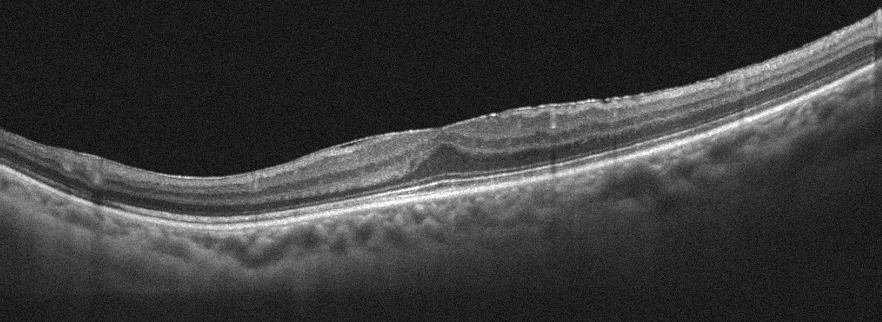
Optical coherence tomography B-scan, fovea-centered, acquired on an Optovue Avanti RTVue XR.
Dx: ERM.